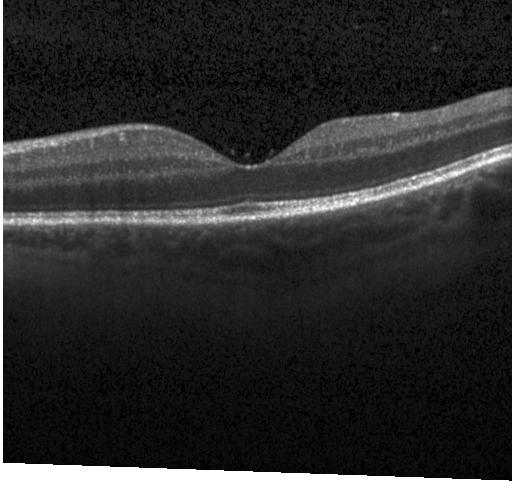

Optical coherence tomography B-scan; instrument: Heidelberg Spectralis; spectral-domain OCT; through the macula.
This B-scan demonstrates no choroidal neovascularization, no diabetic macular edema, and no drusen.